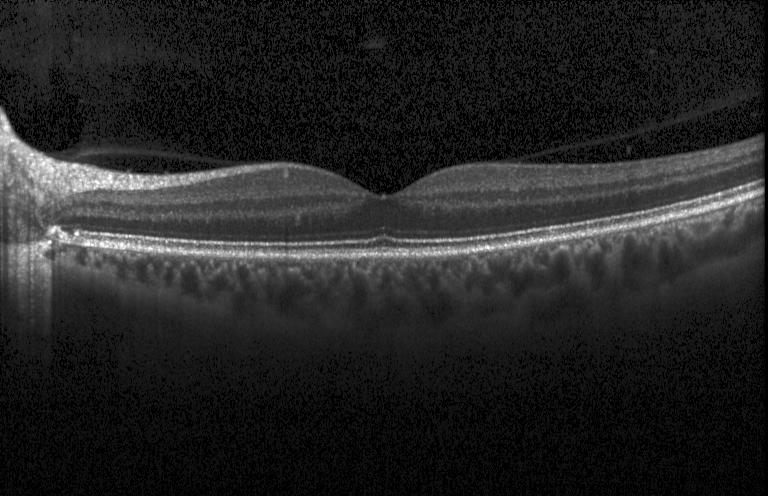

Optical coherence tomography scan, instrument: Heidelberg Spectralis, through the macula
No CNV, no DME, and no drusen.